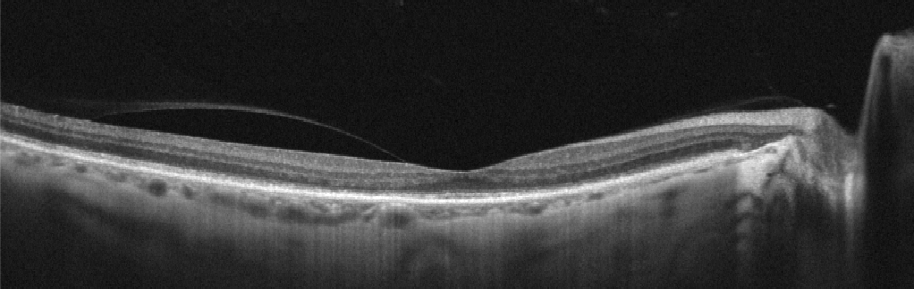
This B-scan demonstrates age-related macular degeneration (AMD).